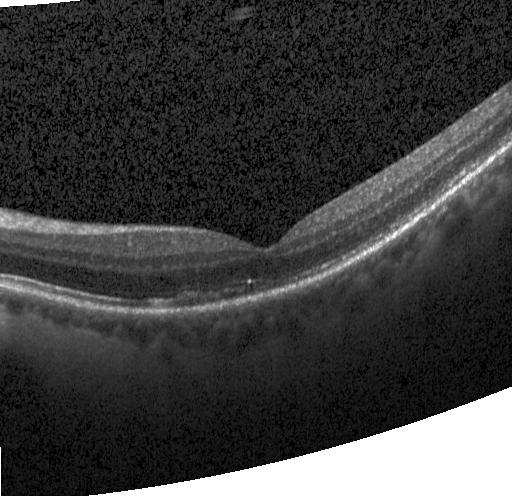

Optical coherence tomography B-scan. SD-OCT. Acquired on a Heidelberg Spectralis.
Diagnosis: no CNV, no DME, and no drusen.